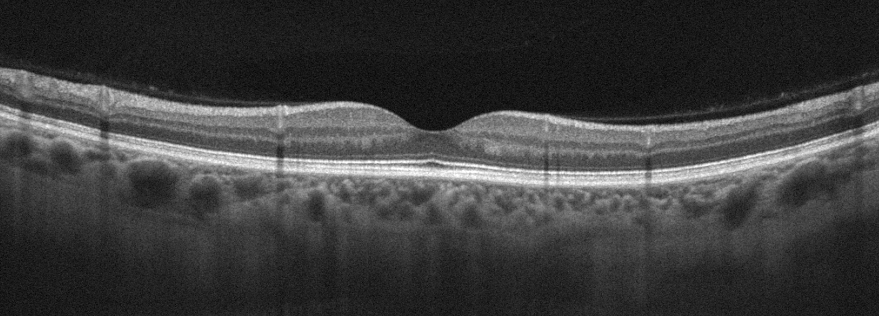

Fovea-centered · optical coherence tomography B-scan
Assessment: no AMD, DME, ERM, RAO, RVO, or VID.